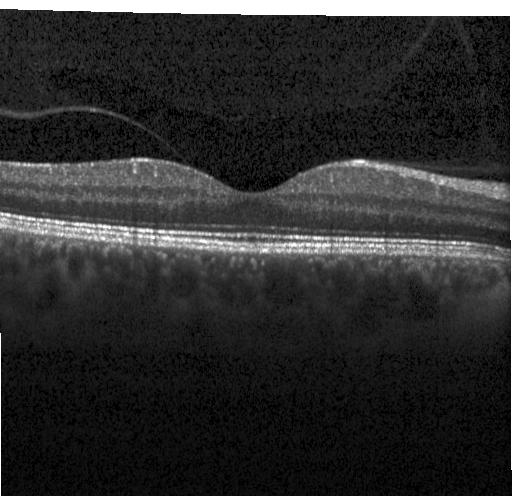 Macular OCT: no CNV, DME, or drusen.